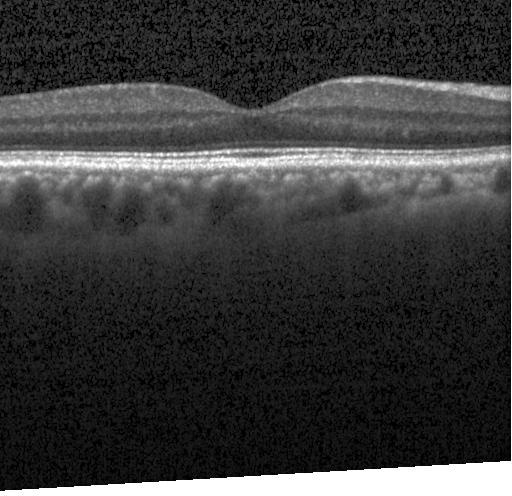
Finding: no evidence of choroidal neovascularization, diabetic macular edema, or drusen.